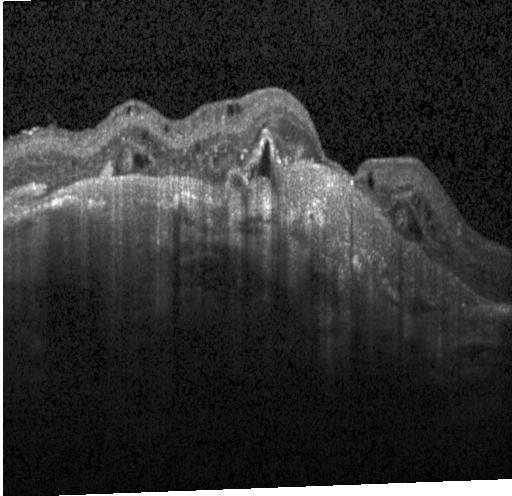
CNV.